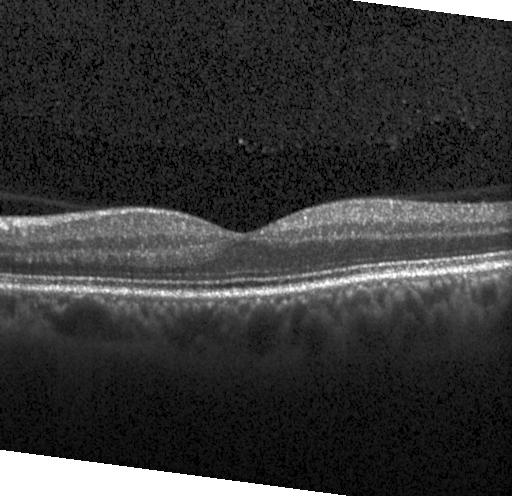

SD-OCT · OCT B-scan · instrument: Heidelberg Spectralis
Impression: no choroidal neovascularization, no diabetic macular edema, and no drusen.